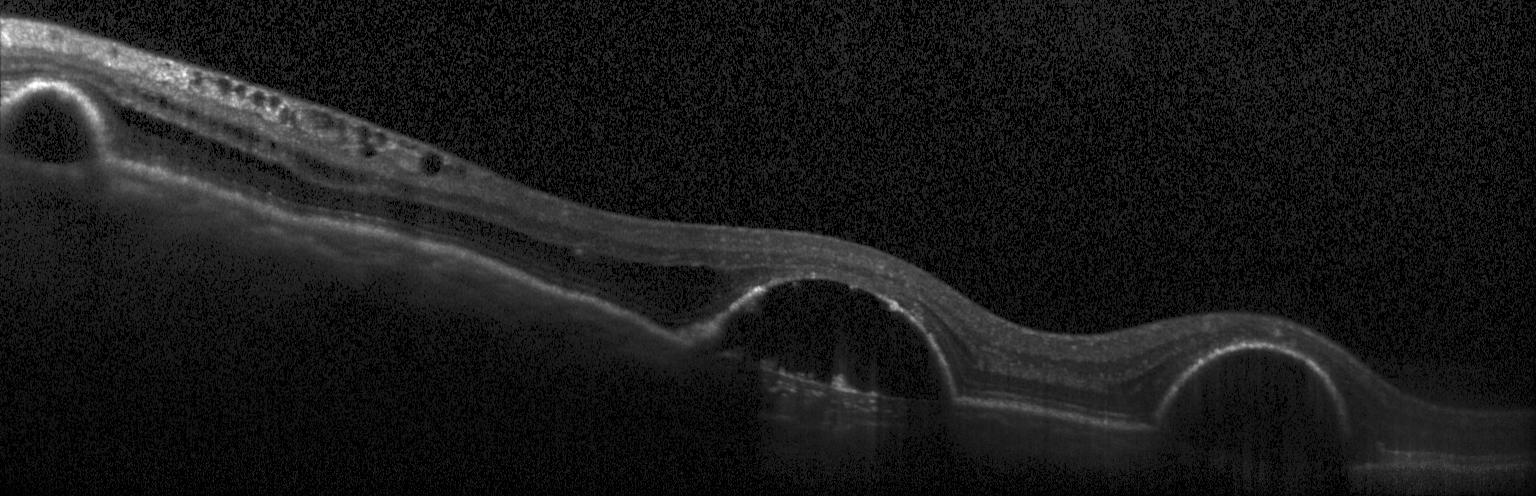

Retinal OCT B-scan — OCT finding: a choroidal neovascular membrane.